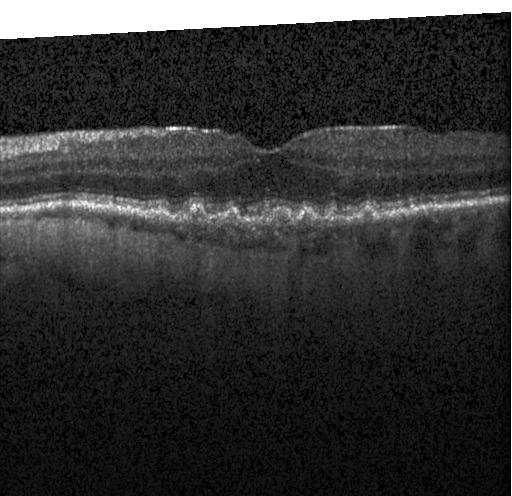 Optical coherence tomography scan; spectral-domain OCT; centered on the fovea — This B-scan demonstrates sub-RPE drusenoid deposits.